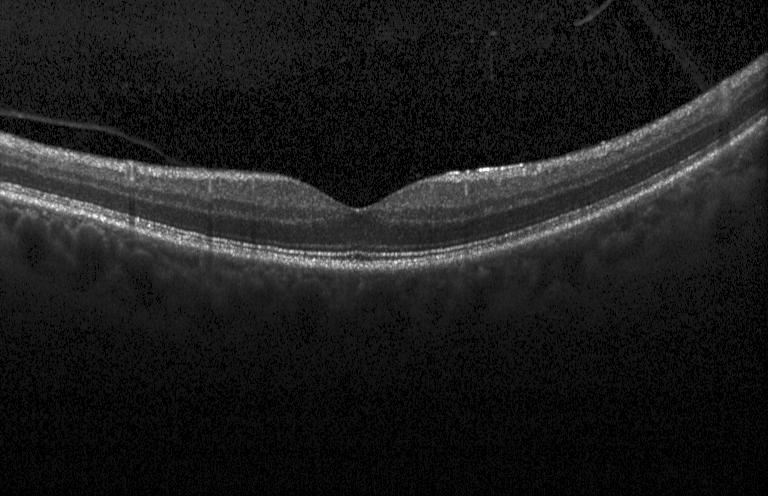
Retinal OCT B-scan; spectral-domain OCT; Heidelberg Spectralis
No choroidal neovascularization, diabetic macular edema, or drusen.